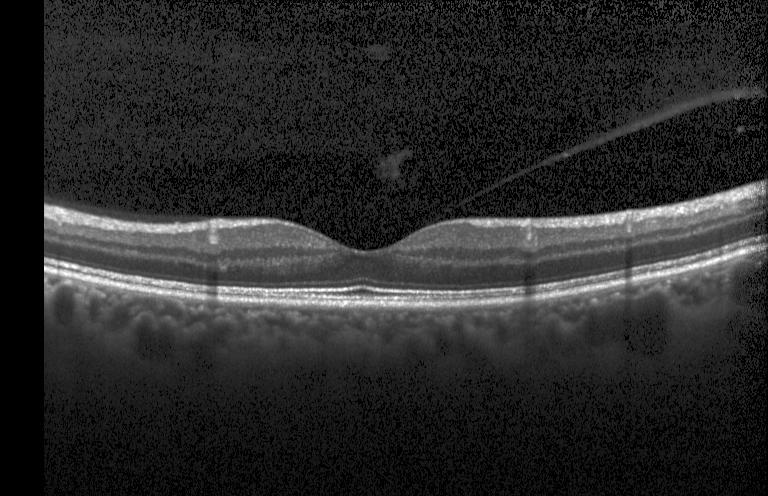

Finding: no choroidal neovascularization, diabetic macular edema, or drusen.